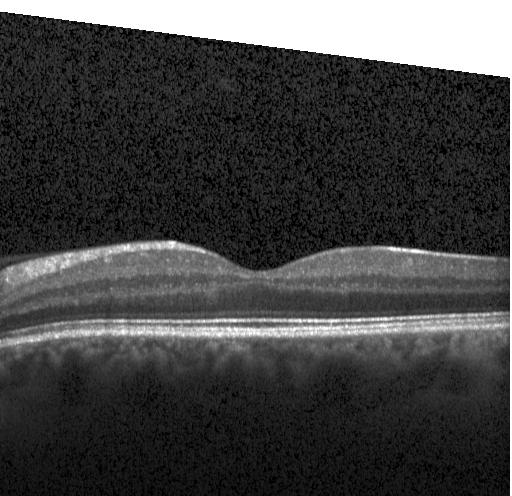
OCT scan showing no CNV, DME, or drusen.